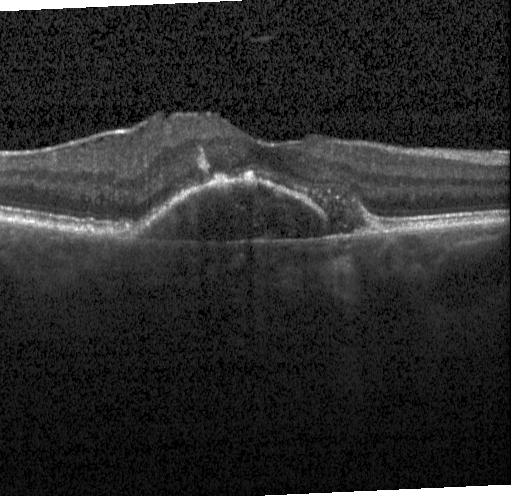

OCT B-scan
Finding: a choroidal neovascular membrane.